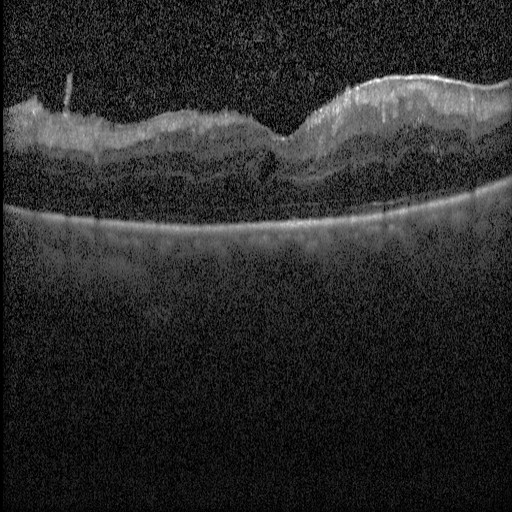 Optical coherence tomography B-scan. Dx: DME.